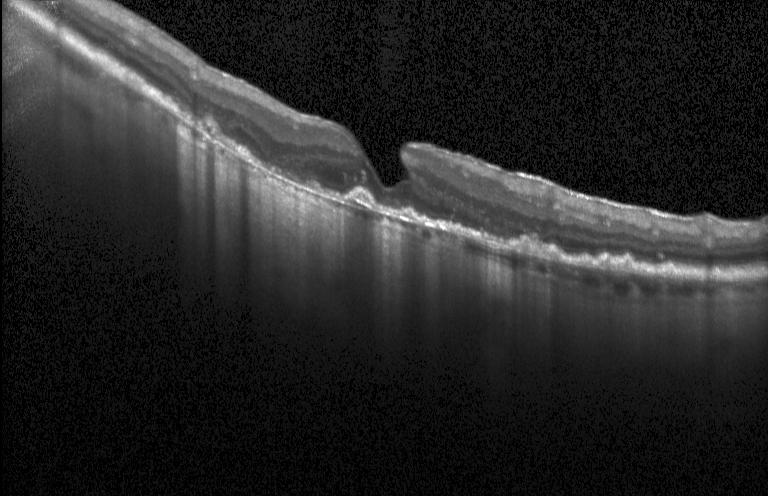 The scan shows a choroidal neovascular membrane.